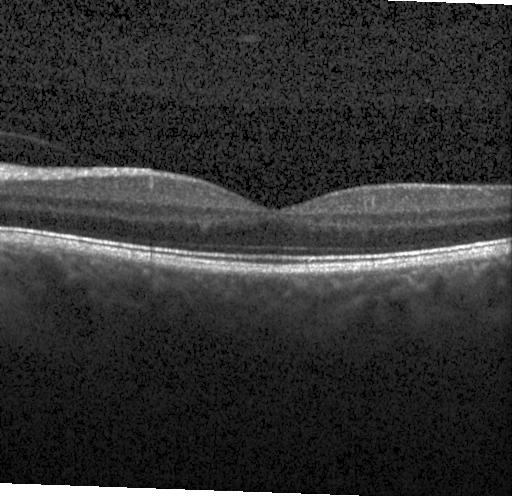

Spectral-domain OCT B-scan: neither choroidal neovascularization, diabetic macular edema, nor drusen.